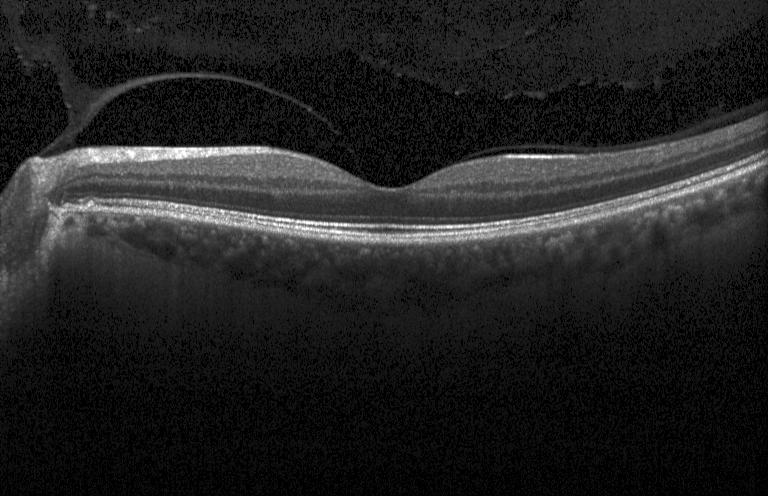 OCT B-scan.
This B-scan demonstrates no evidence of CNV, DME, or drusen.